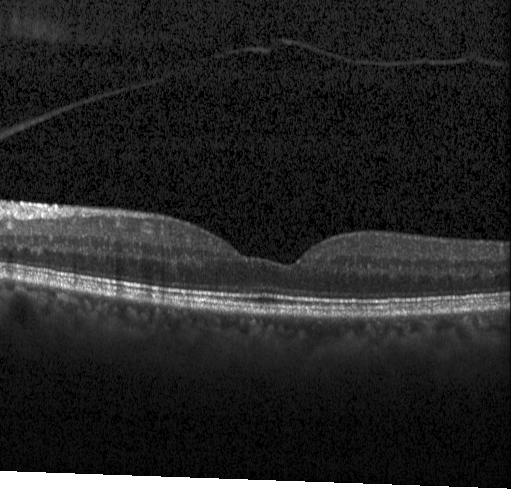
Finding: neither CNV, DME, nor drusen.